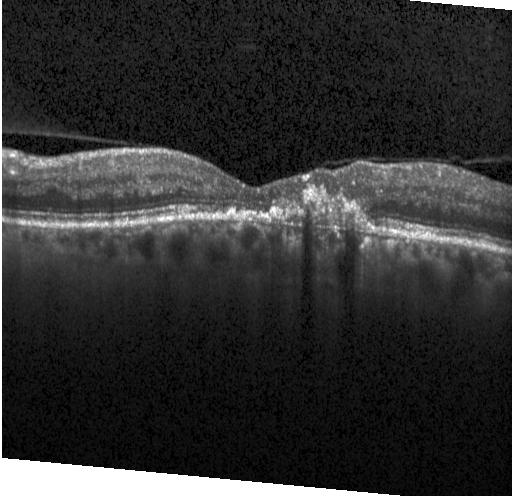

Fovea-centered · acquired on a Heidelberg Spectralis · retinal OCT cross-section · spectral-domain optical coherence tomography.
This B-scan demonstrates CNV.